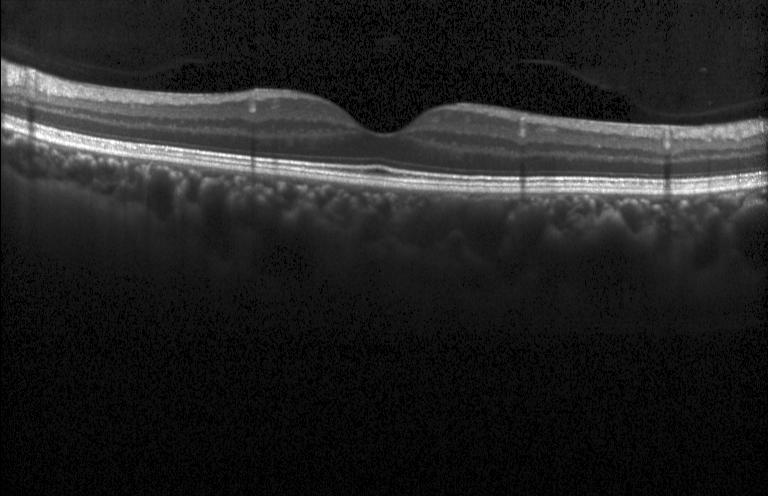

Macular scan · SD-OCT · retinal OCT cross-section. This B-scan demonstrates no evidence of choroidal neovascularization, diabetic macular edema, or drusen.